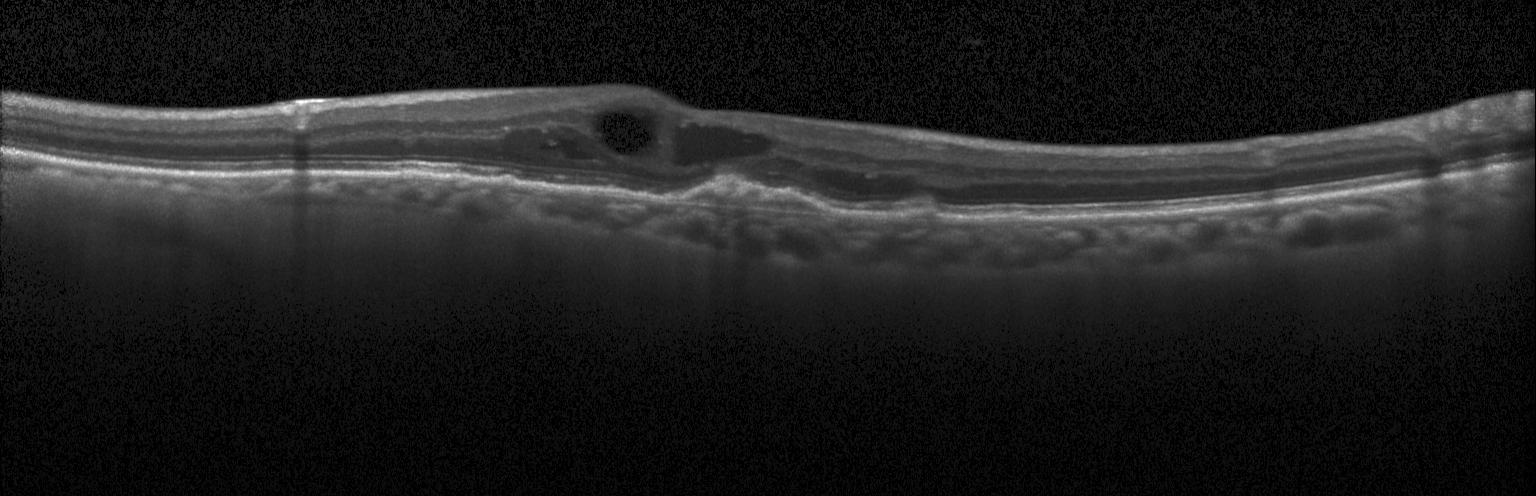

OCT B-scan · Heidelberg Spectralis.
This B-scan demonstrates a choroidal neovascular membrane.